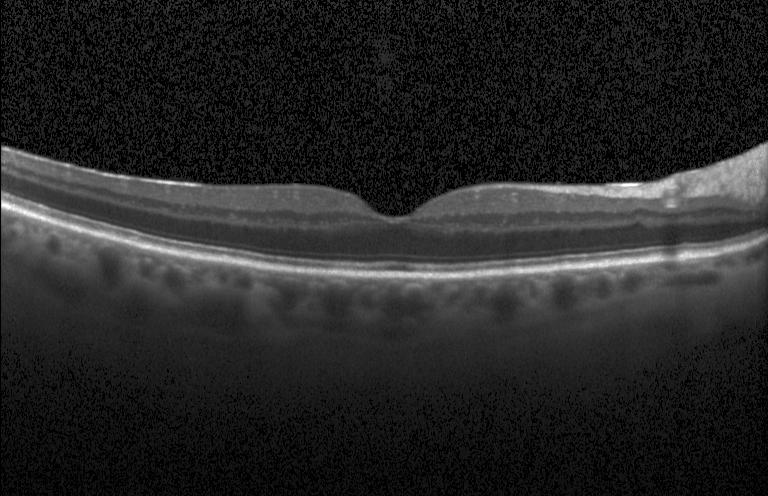
Retinal OCT B-scan; macular scan; SD-OCT; instrument: Heidelberg Spectralis
This B-scan demonstrates no choroidal neovascularization, diabetic macular edema, or drusen.